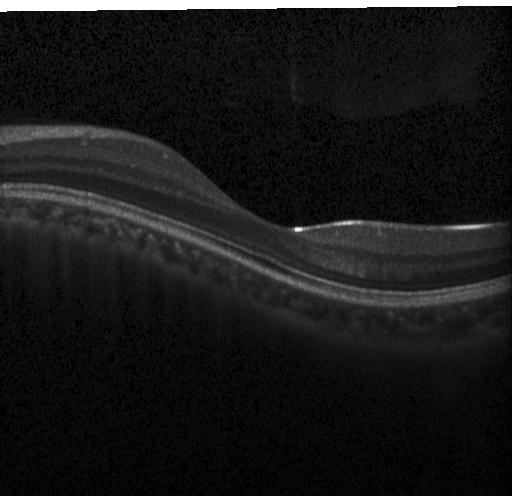 Fovea-centered, OCT line scan, spectral-domain optical coherence tomography, instrument: Heidelberg Spectralis
No evidence of choroidal neovascularization, diabetic macular edema, or drusen.